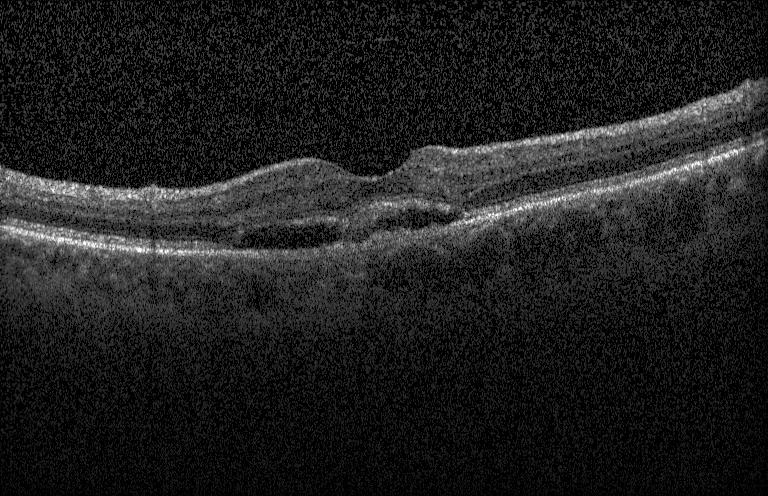
Diagnosis: a choroidal neovascular membrane.